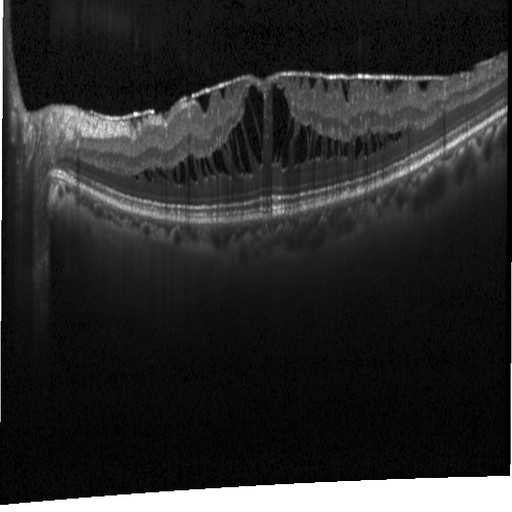 Retinal OCT B-scan
OCT finding: DME.